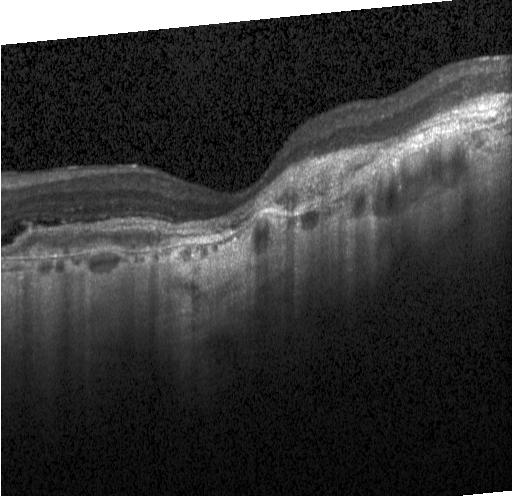
Macular OCT: a choroidal neovascular membrane.